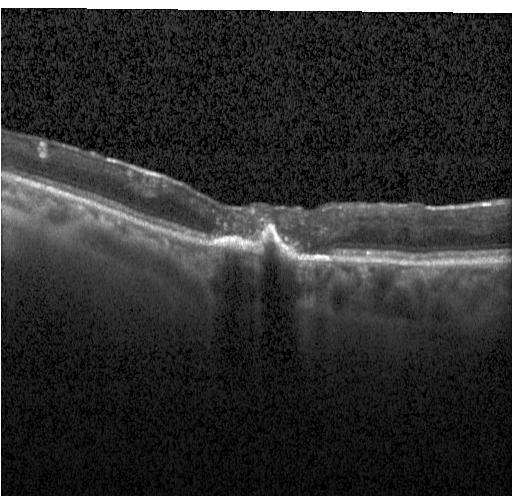

Impression: CNV.